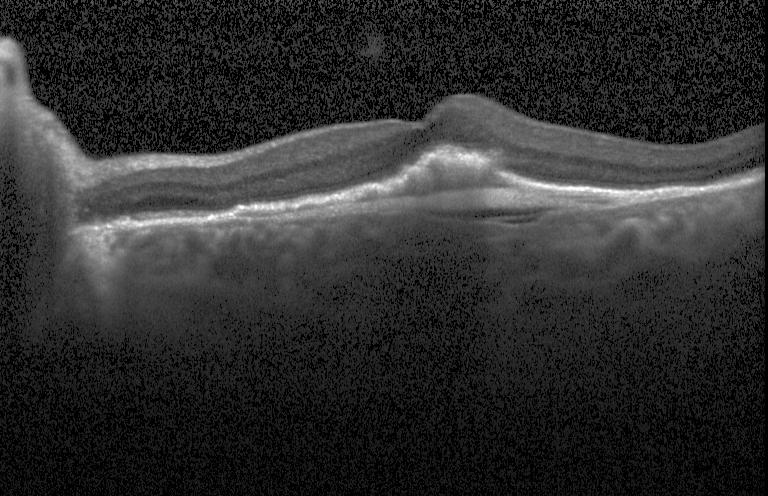
Optical coherence tomography B-scan, fovea-centered
A choroidal neovascular membrane.